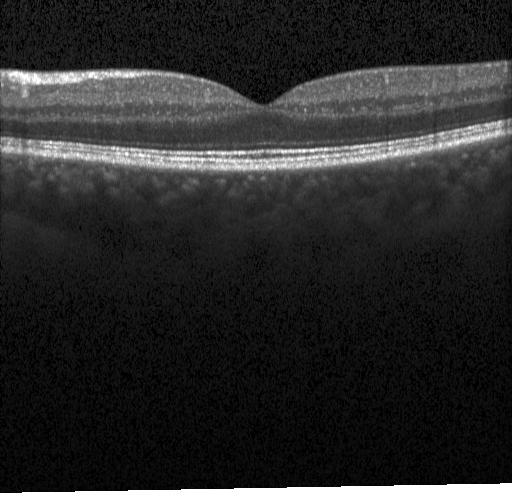 Macular OCT demonstrating no choroidal neovascularization, no diabetic macular edema, and no drusen.